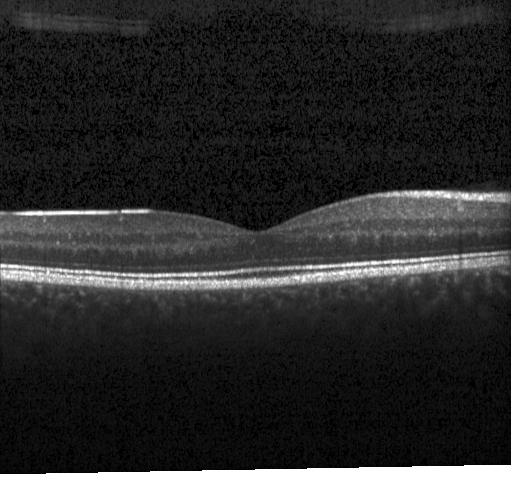
Finding: no evidence of choroidal neovascularization, diabetic macular edema, or drusen.